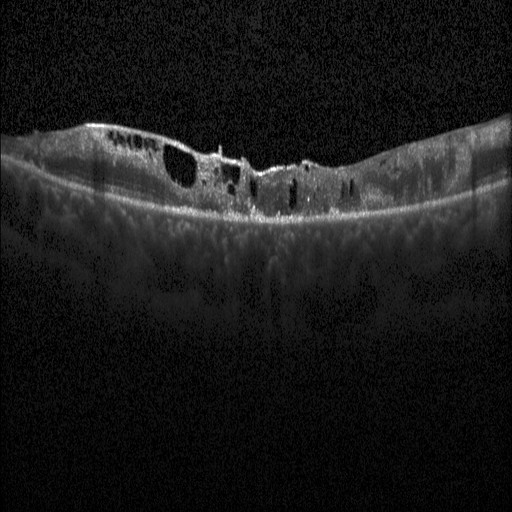
Centered on the fovea; optical coherence tomography scan; spectral-domain OCT
OCT finding: DME.